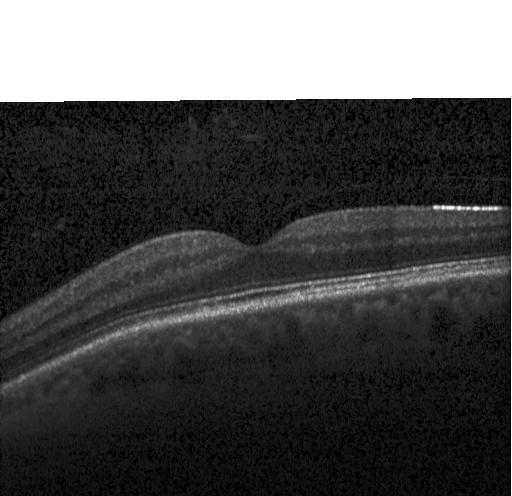
Horizontal scan through the fovea · OCT line scan · instrument: Heidelberg Spectralis. Assessment: neither choroidal neovascularization, diabetic macular edema, nor drusen.